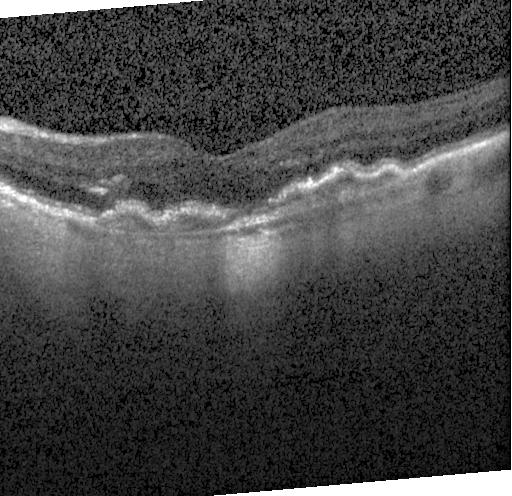

Acquired on a Heidelberg Spectralis · retinal OCT B-scan · horizontal scan through the fovea.
Diagnosis: a choroidal neovascular membrane.